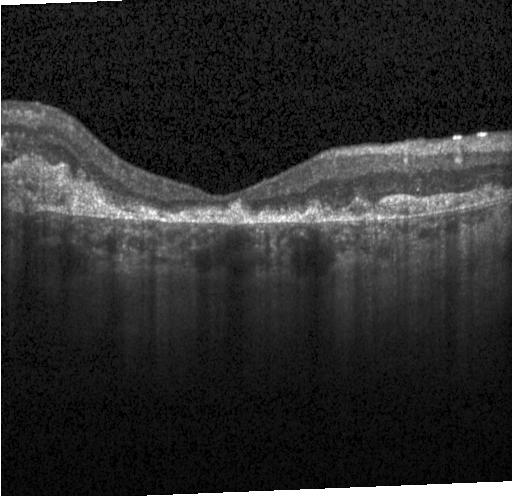

OCT scan showing choroidal neovascularization.